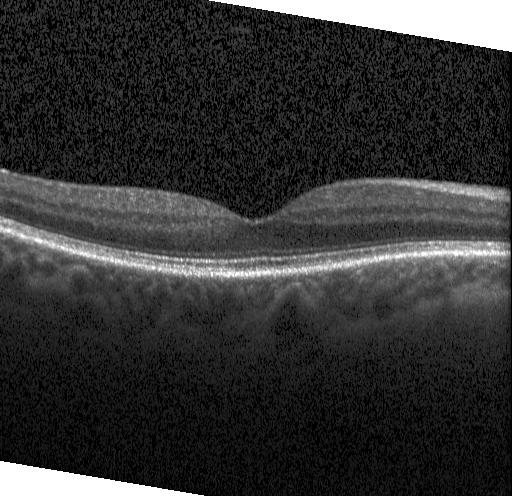
Spectral-domain OCT, through the macula, OCT B-scan, acquired on a Heidelberg Spectralis. Finding: no choroidal neovascularization, diabetic macular edema, or drusen.